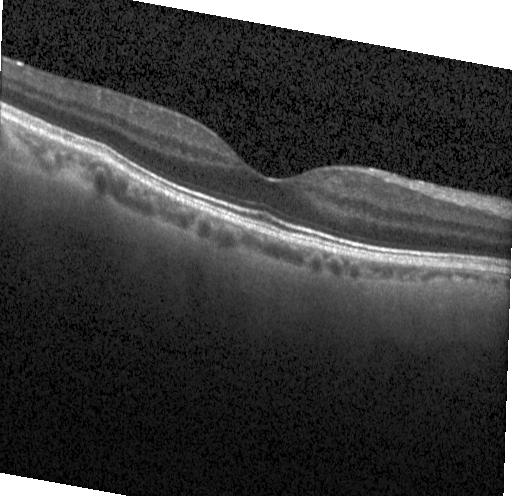 Heidelberg Spectralis. Optical coherence tomography scan.
Finding: no evidence of choroidal neovascularization, diabetic macular edema, or drusen.